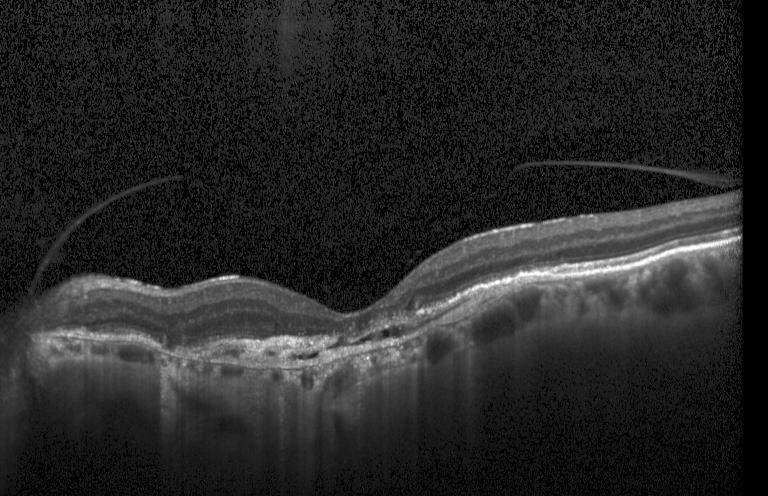
Optical coherence tomography B-scan; Heidelberg Spectralis OCT system; spectral-domain optical coherence tomography; macular scan.
Diagnosis: choroidal neovascularization (CNV).